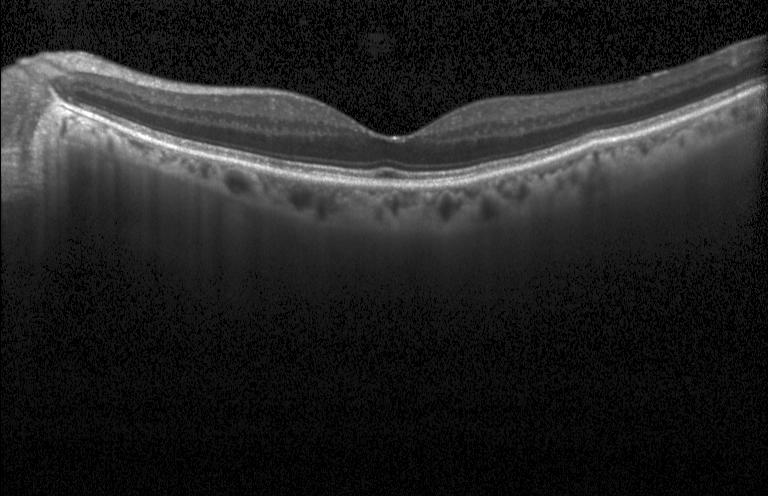

No choroidal neovascularization, no diabetic macular edema, and no drusen.